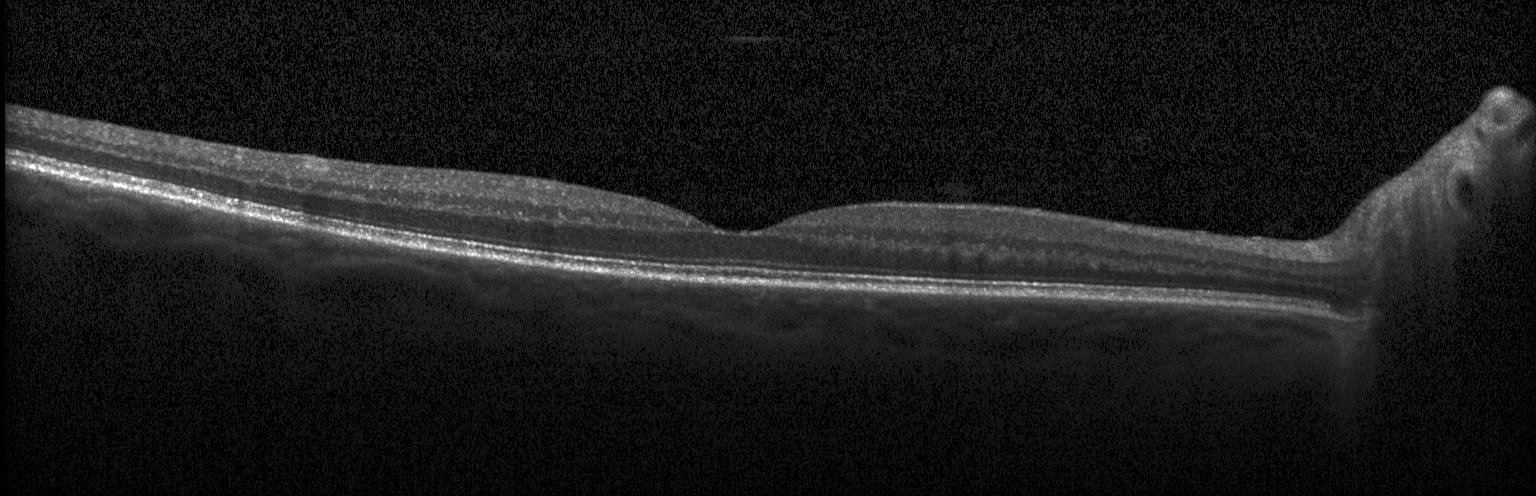

OCT B-scan showing no choroidal neovascularization, no diabetic macular edema, and no drusen.